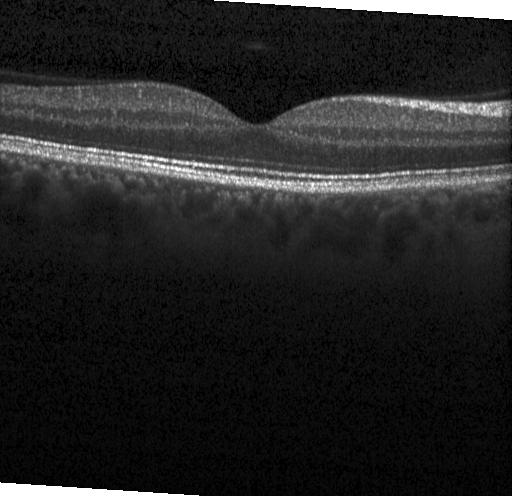

Acquired on a Heidelberg Spectralis · macular scan · OCT line scan — OCT finding: neither choroidal neovascularization, diabetic macular edema, nor drusen.